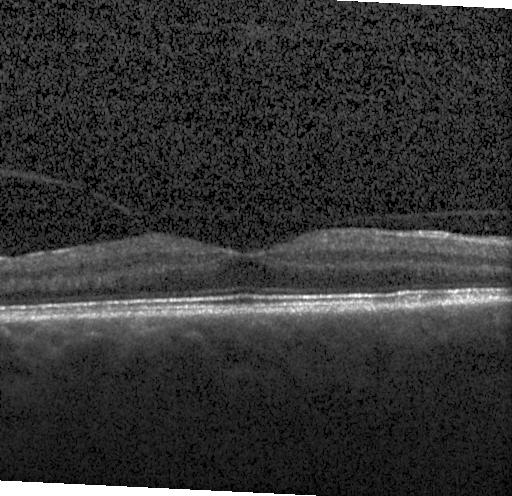

Instrument: Heidelberg Spectralis, OCT B-scan, fovea-centered, SD-OCT.
Assessment: neither choroidal neovascularization, diabetic macular edema, nor drusen.